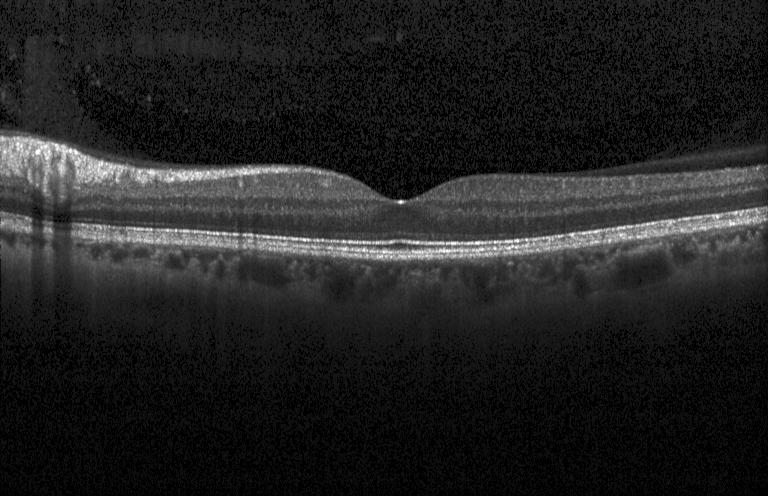

Heidelberg Spectralis. OCT B-scan. Centered on the fovea.
Finding: no choroidal neovascularization, no diabetic macular edema, and no drusen.